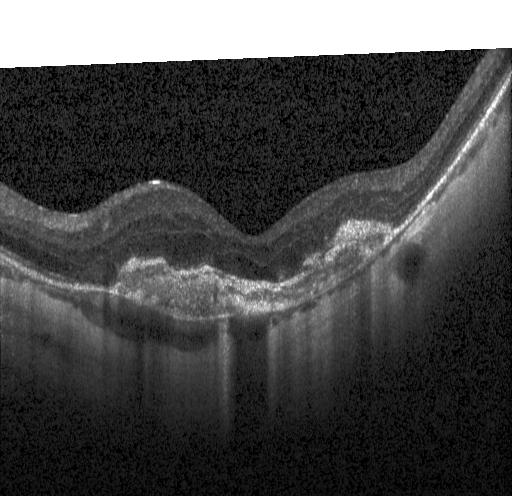

Fovea-centered · spectral-domain OCT · instrument: Heidelberg Spectralis · OCT B-scan
The scan shows choroidal neovascularization (CNV).